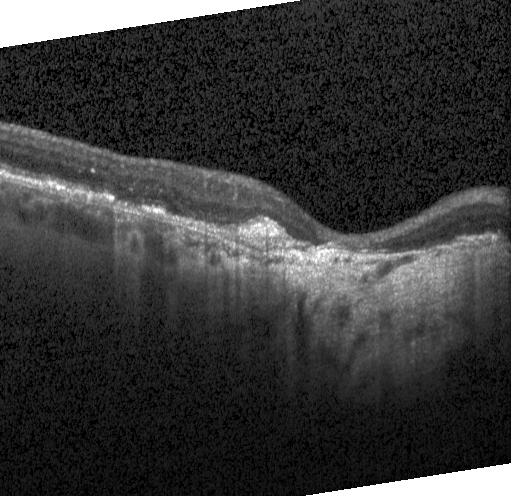 OCT line scan, SD-OCT
This B-scan demonstrates a choroidal neovascular membrane.